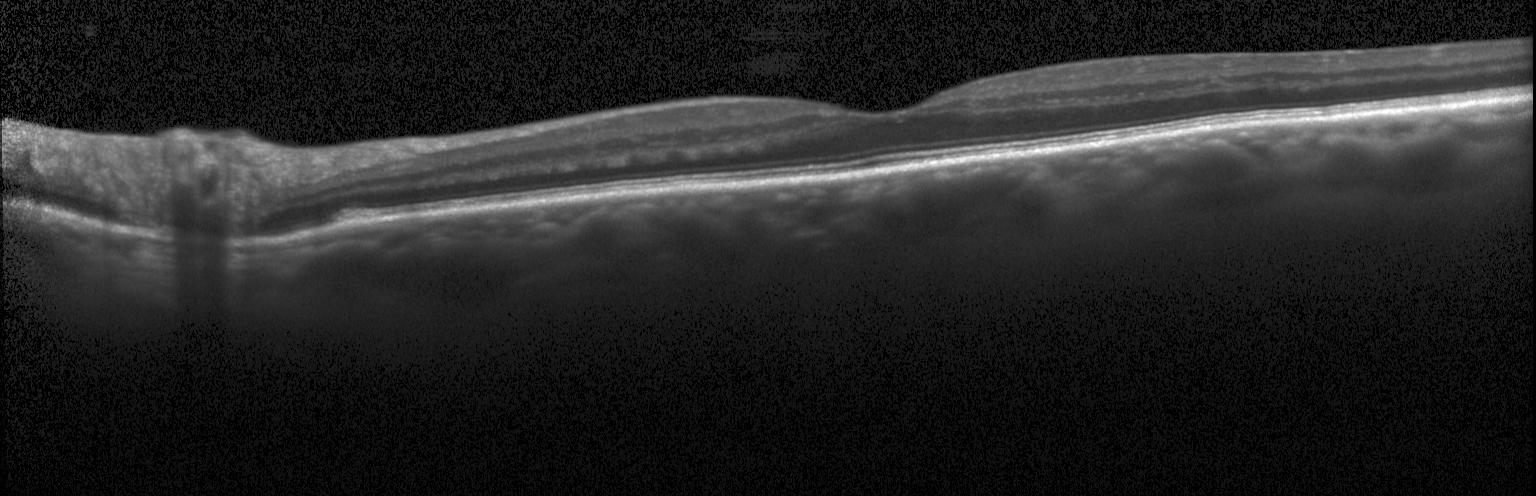

Fovea-centered · instrument: Heidelberg Spectralis · OCT B-scan · spectral-domain OCT. Finding: no choroidal neovascularization, no diabetic macular edema, and no drusen.